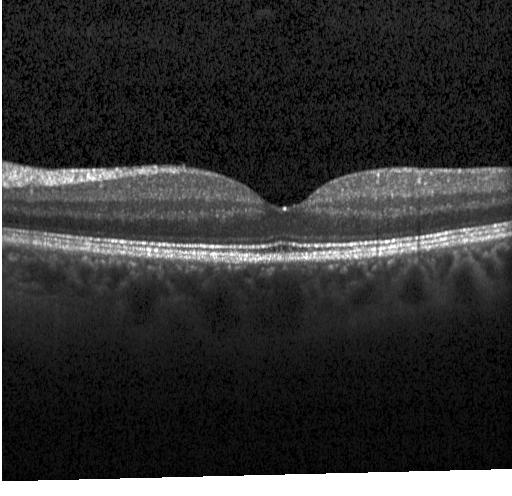

SD-OCT. OCT line scan.
Impression: no evidence of choroidal neovascularization, diabetic macular edema, or drusen.